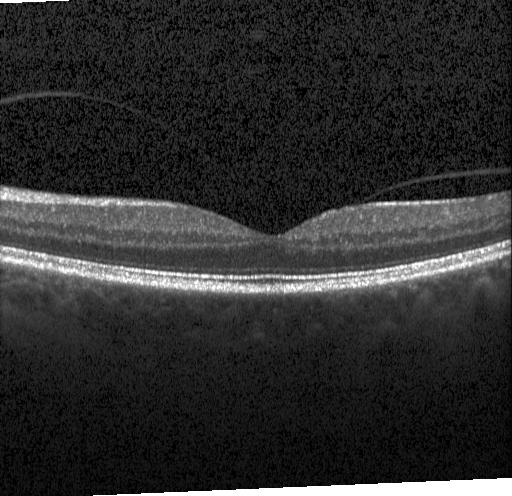

Finding: no evidence of choroidal neovascularization, diabetic macular edema, or drusen.